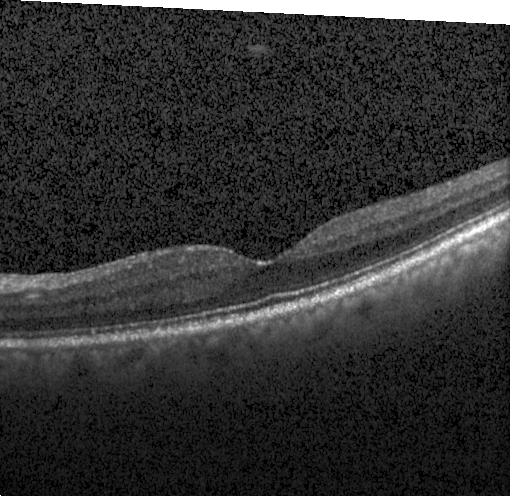 Dx: no choroidal neovascularization, diabetic macular edema, or drusen.